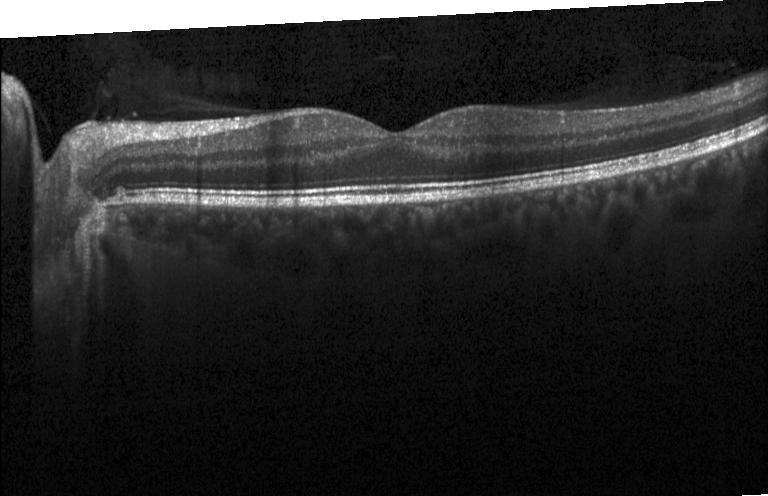

This B-scan demonstrates neither CNV, DME, nor drusen.